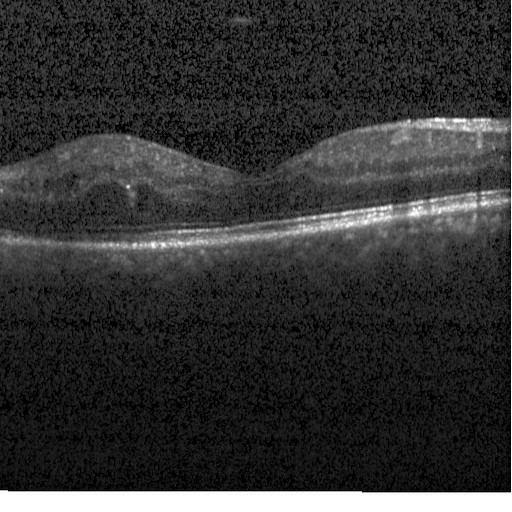

Assessment: DME.